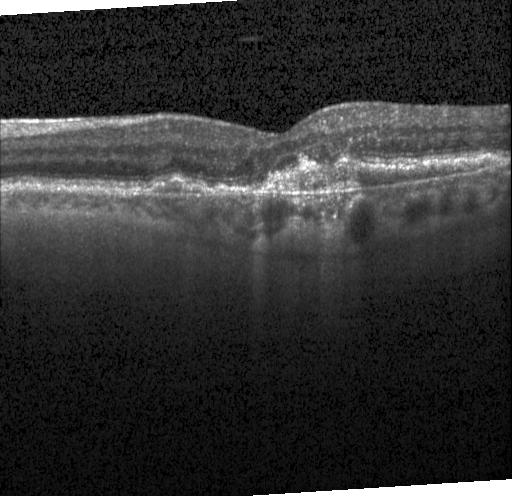

Heidelberg Spectralis · retinal OCT cross-section · spectral-domain OCT — Dx: CNV.